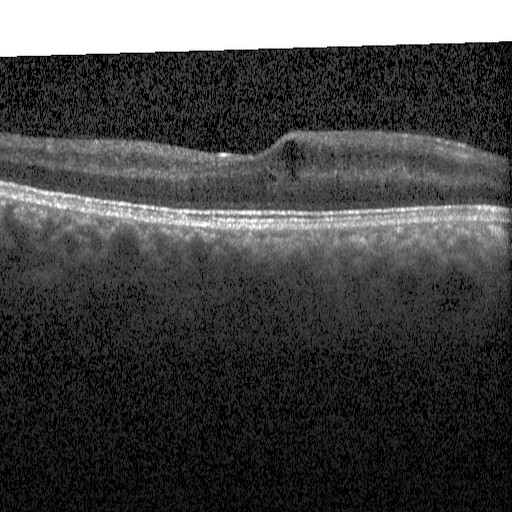 Finding: DME.